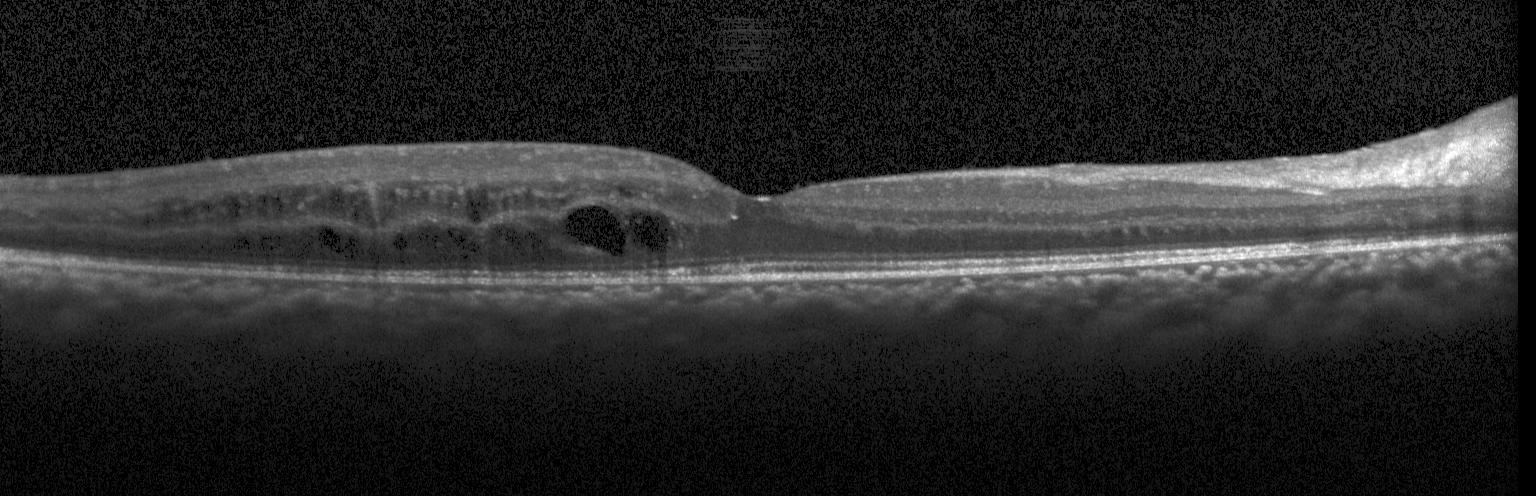

Impression: diabetic macular edema (DME).